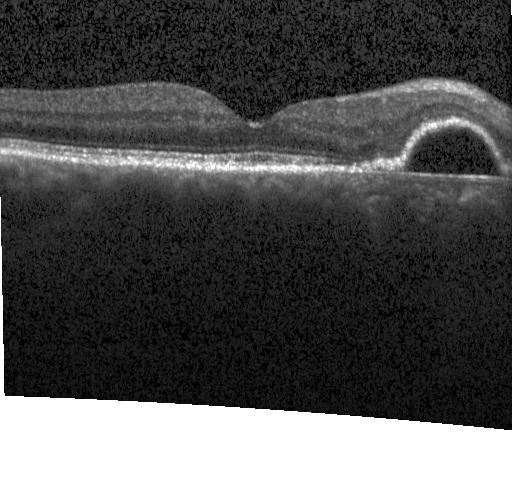
SD-OCT, horizontal scan through the fovea, acquired on a Heidelberg Spectralis, retinal OCT B-scan. Finding: CNV.